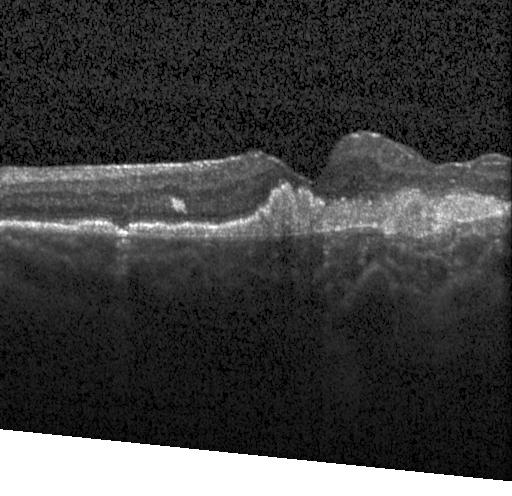

Diagnosis: choroidal neovascularization.